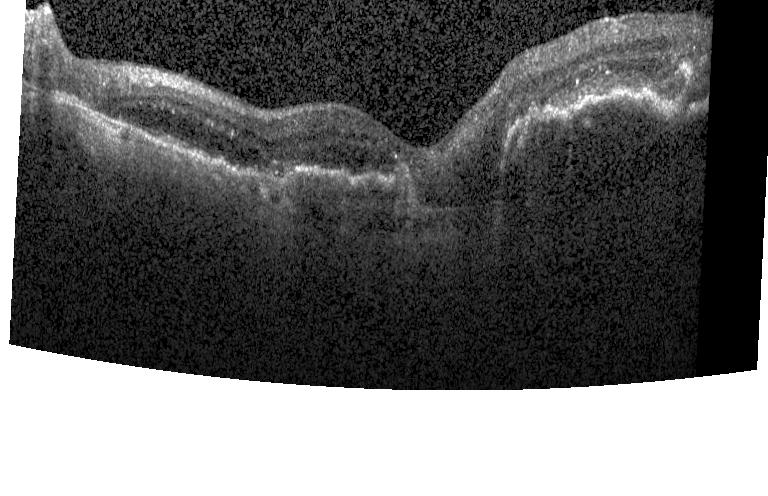
Retinal OCT cross-section showing choroidal neovascularization.